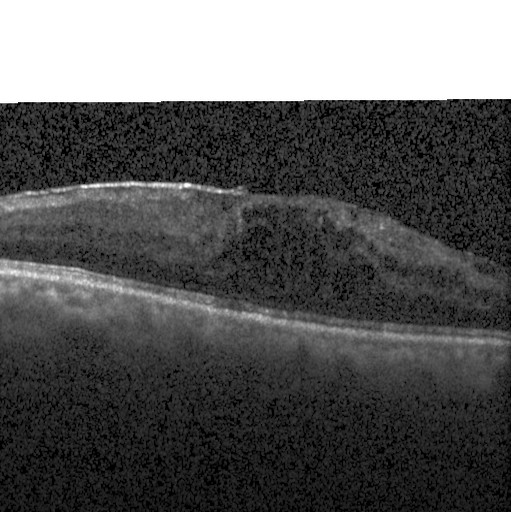

Optical coherence tomography B-scan. Spectral-domain OCT. Instrument: Heidelberg Spectralis. Centered on the fovea
Finding: diabetic macular edema (DME).